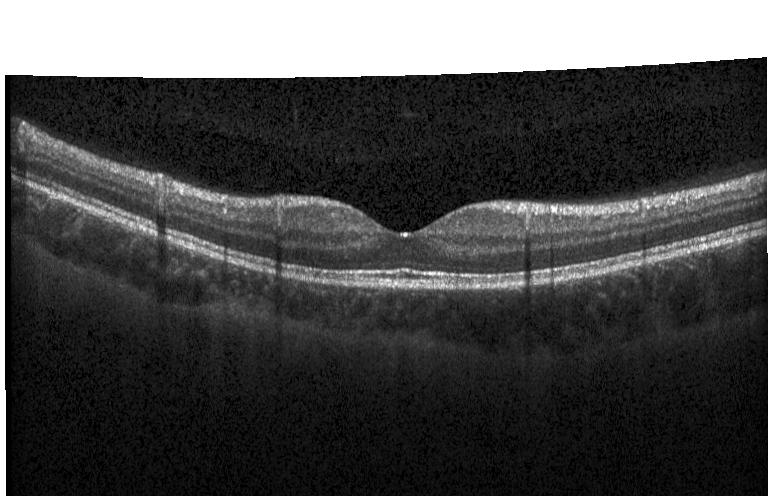

OCT line scan — Assessment: neither choroidal neovascularization, diabetic macular edema, nor drusen.